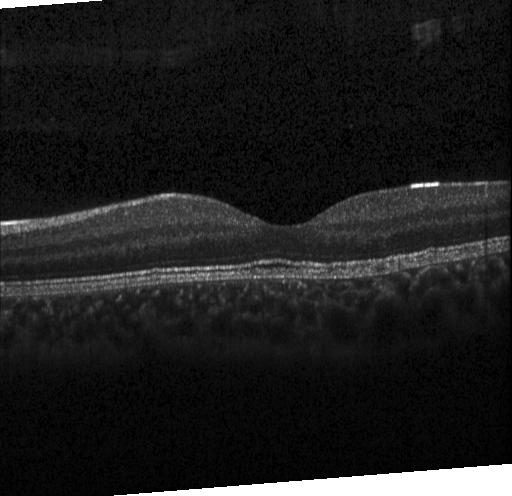
Optical coherence tomography B-scan, Heidelberg Spectralis OCT system, horizontal scan through the fovea
Finding: neither CNV, DME, nor drusen.